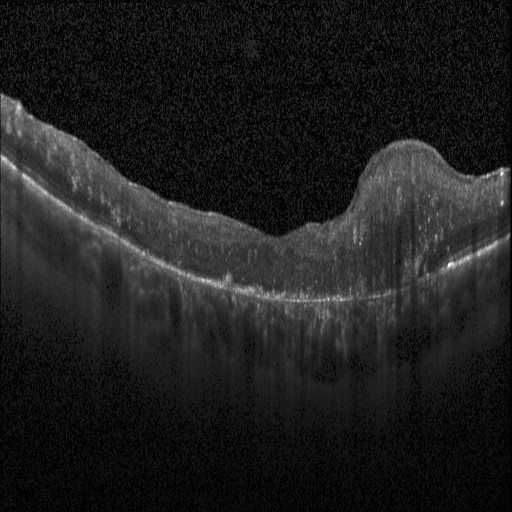 Impression: DME.